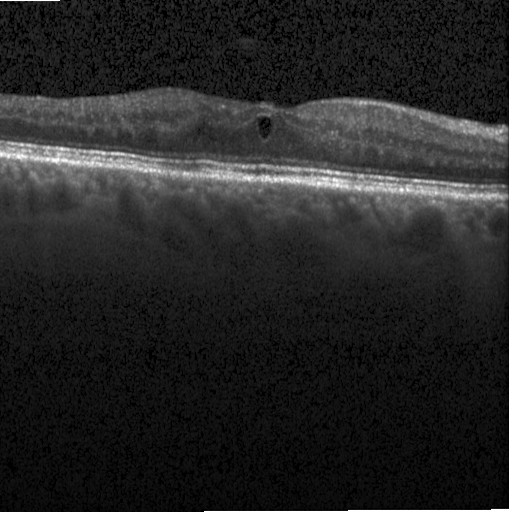
Retinal OCT cross-section
Diagnosis: diabetic macular edema.